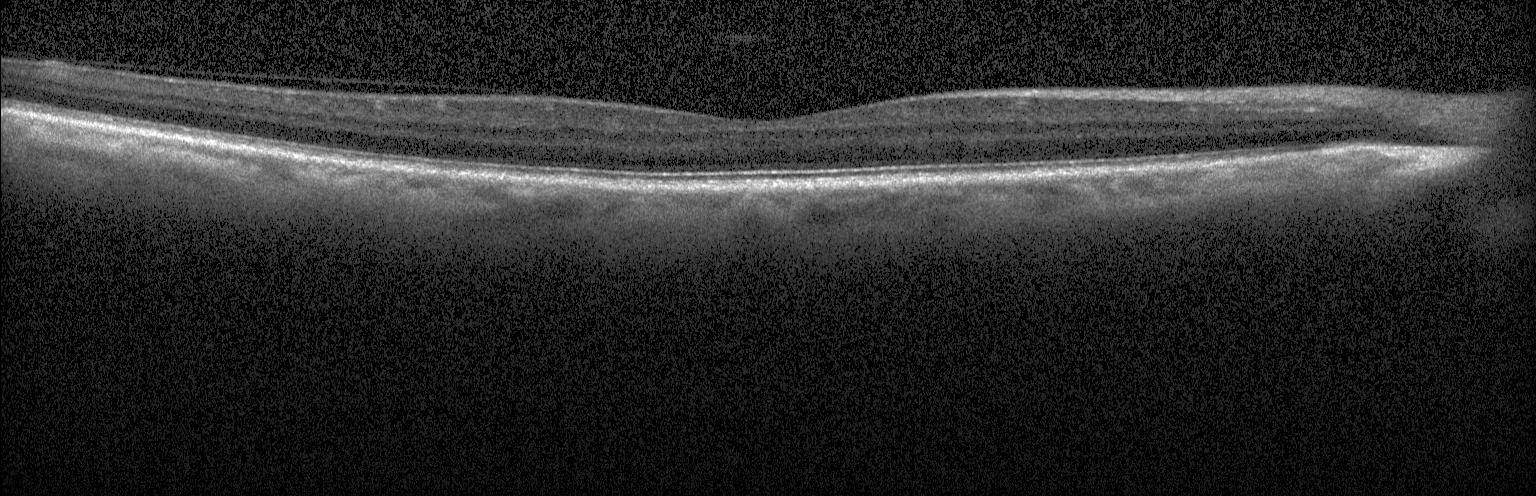

Spectral-domain OCT, OCT B-scan, Heidelberg Spectralis, centered on the fovea — Impression: no choroidal neovascularization, diabetic macular edema, or drusen.